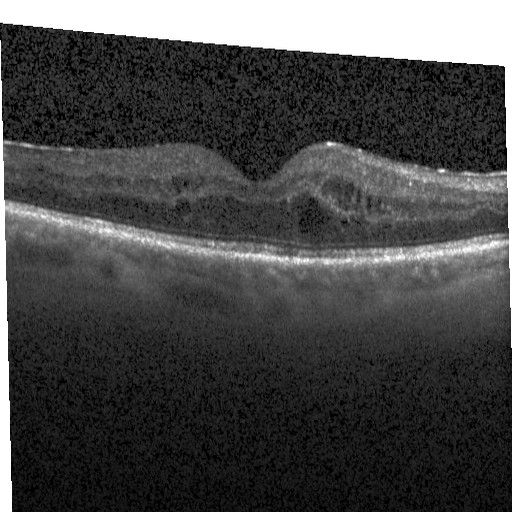
Optical coherence tomography scan — Finding: diabetic macular edema (DME).